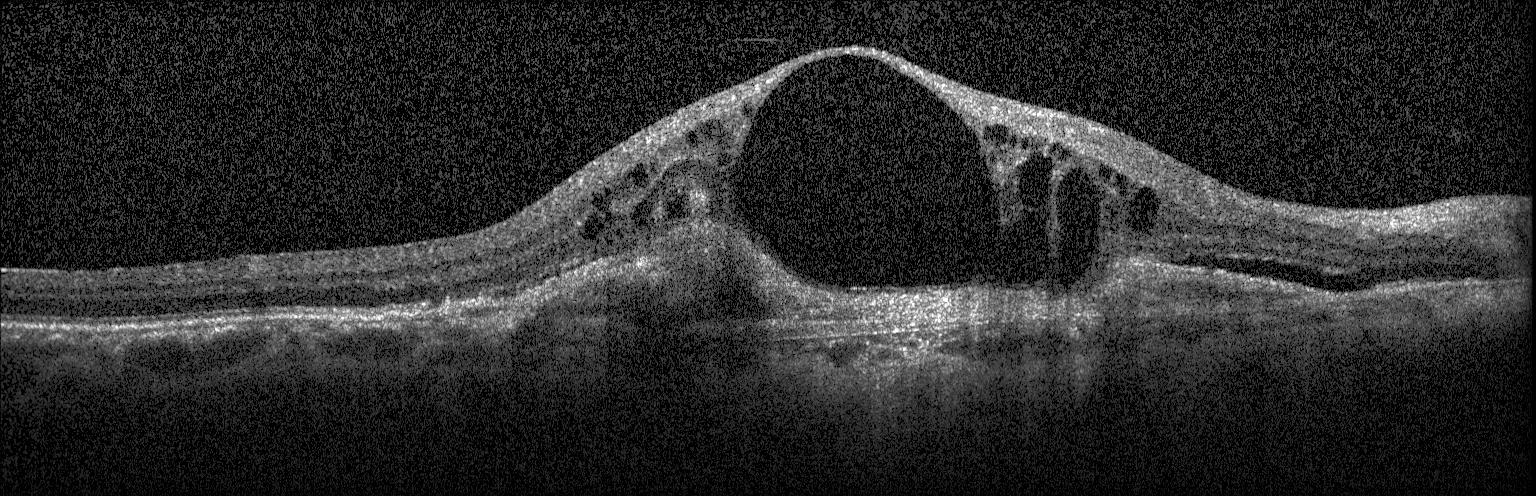 Retinal OCT cross-section showing a choroidal neovascular membrane.